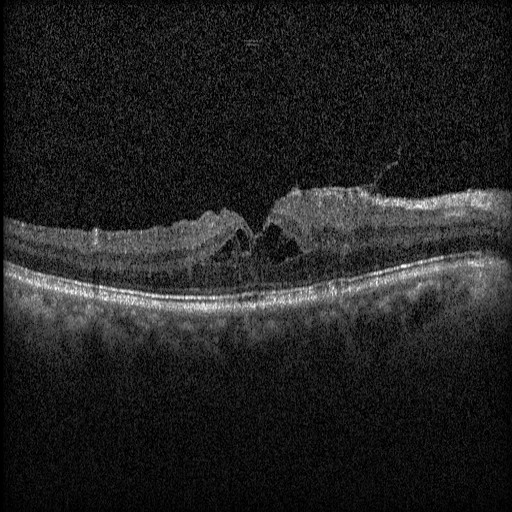 SD-OCT, acquired on a Heidelberg Spectralis, retinal OCT B-scan
Assessment: diabetic macular edema (DME).